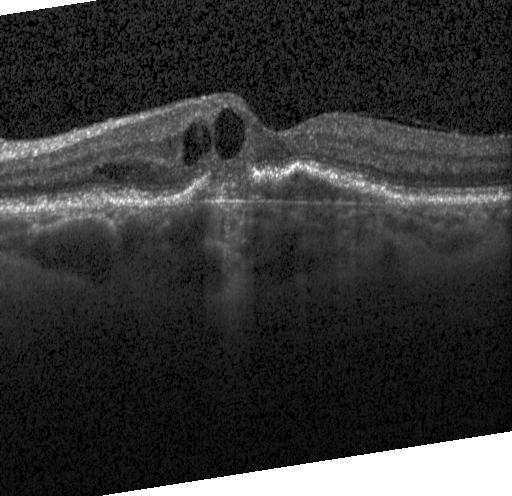 Spectral-domain optical coherence tomography · Heidelberg Spectralis OCT system · OCT B-scan. Diagnosis: a choroidal neovascular membrane.